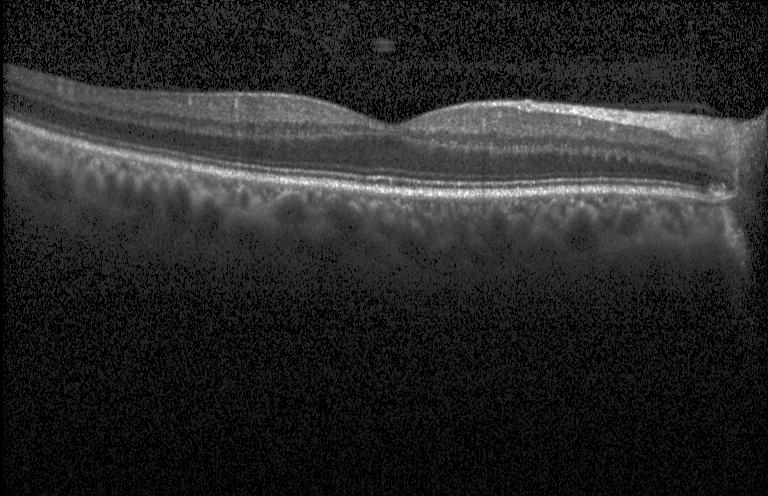

OCT B-scan.
Macular OCT: neither choroidal neovascularization, diabetic macular edema, nor drusen.